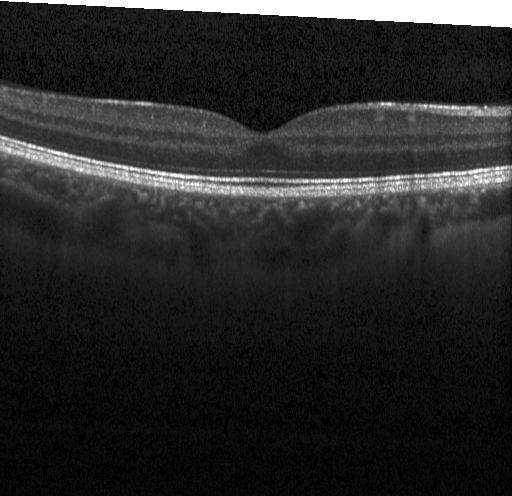
The scan shows no choroidal neovascularization, no diabetic macular edema, and no drusen.